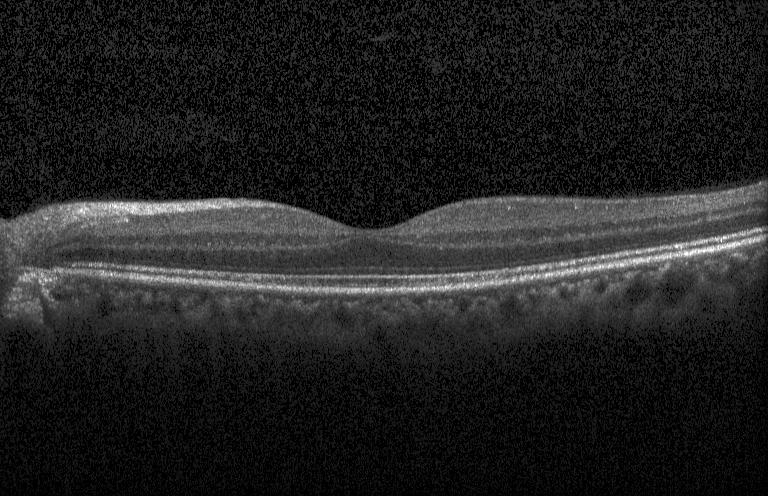

OCT line scan. Through the macula.
OCT finding: neither choroidal neovascularization, diabetic macular edema, nor drusen.